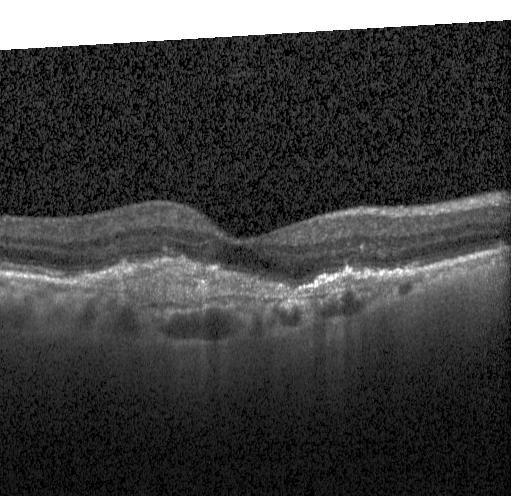 Dx: choroidal neovascularization.